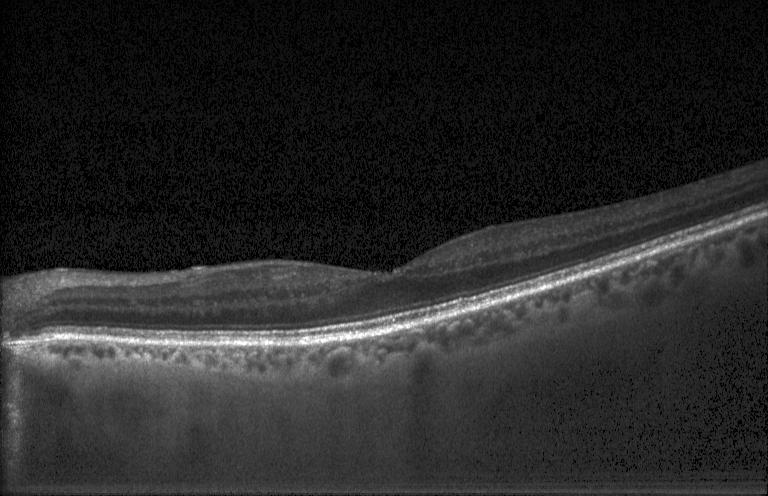 Optical coherence tomography B-scan
The scan shows no CNV, DME, or drusen.